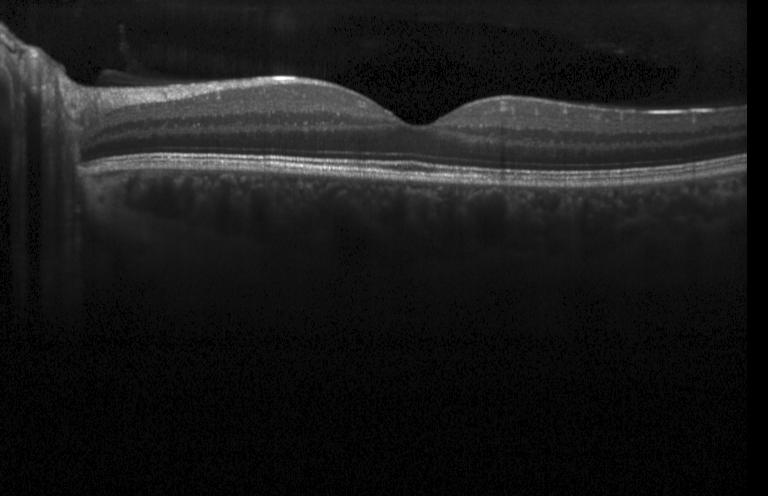 Optical coherence tomography scan. Finding: no choroidal neovascularization, diabetic macular edema, or drusen.